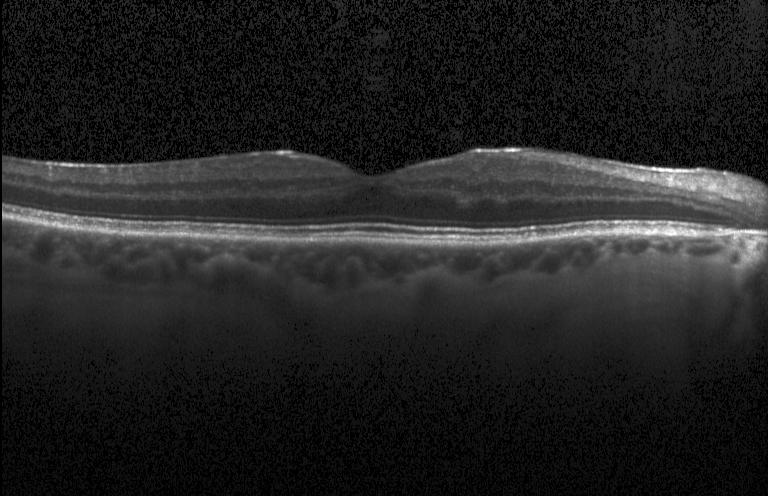 Retinal OCT B-scan, fovea-centered, spectral-domain optical coherence tomography, acquired on a Heidelberg Spectralis.
The scan shows no choroidal neovascularization, no diabetic macular edema, and no drusen.